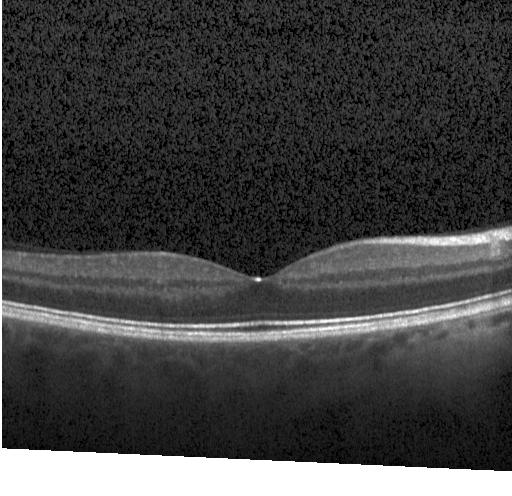 Macular scan. Heidelberg Spectralis. Optical coherence tomography scan. Spectral-domain OCT
No evidence of CNV, DME, or drusen.